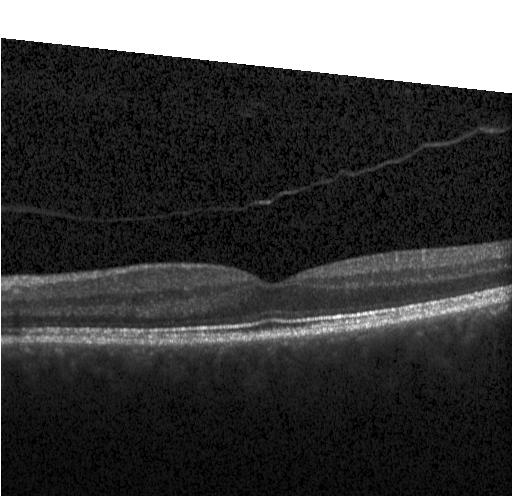

Finding: no choroidal neovascularization, no diabetic macular edema, and no drusen.